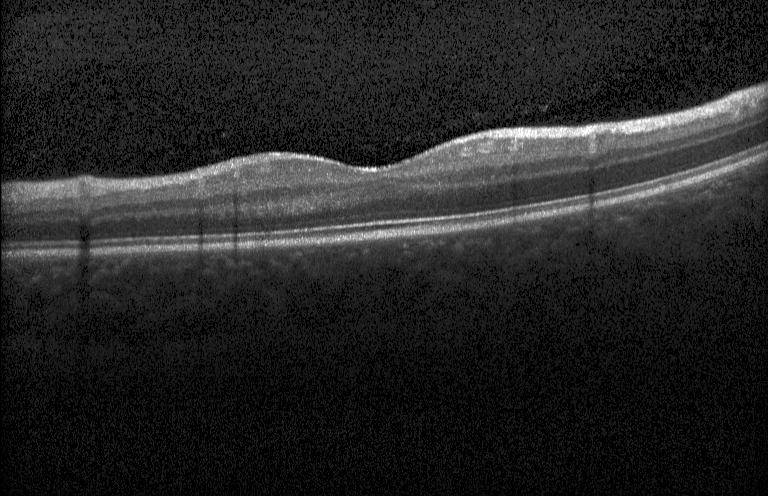
Retinal OCT B-scan — Diagnosis: neither choroidal neovascularization, diabetic macular edema, nor drusen.